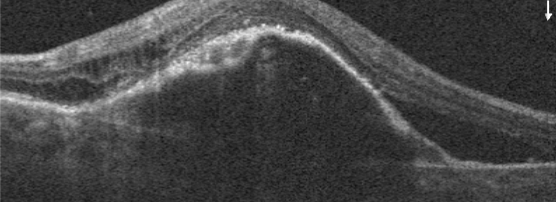
Instrument: Optovue Avanti RTVue XR. Optical coherence tomography B-scan. Assessment: age-related macular degeneration (AMD).